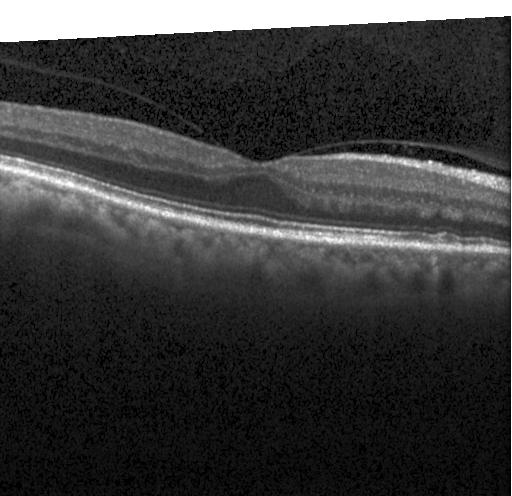
Finding: sub-RPE drusenoid deposits.